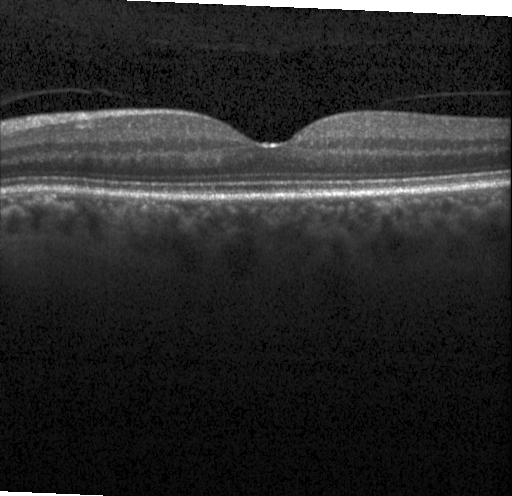

This B-scan demonstrates no evidence of choroidal neovascularization, diabetic macular edema, or drusen.